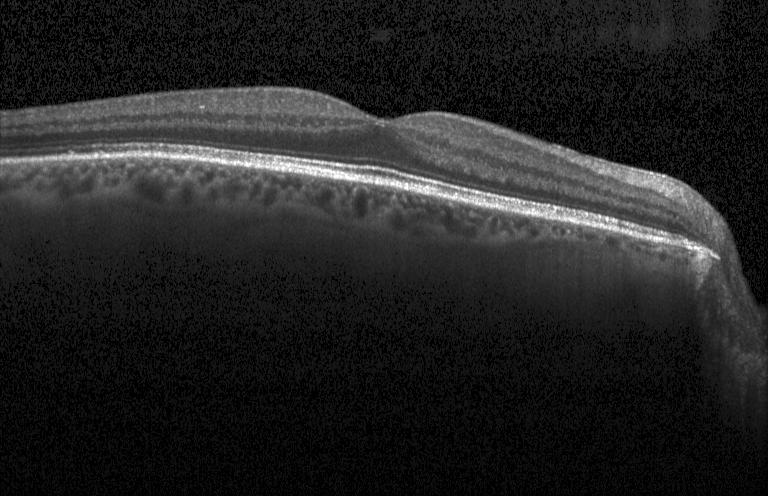 Optical coherence tomography scan, macular scan, spectral-domain OCT, Heidelberg Spectralis OCT system. Finding: no choroidal neovascularization, diabetic macular edema, or drusen.